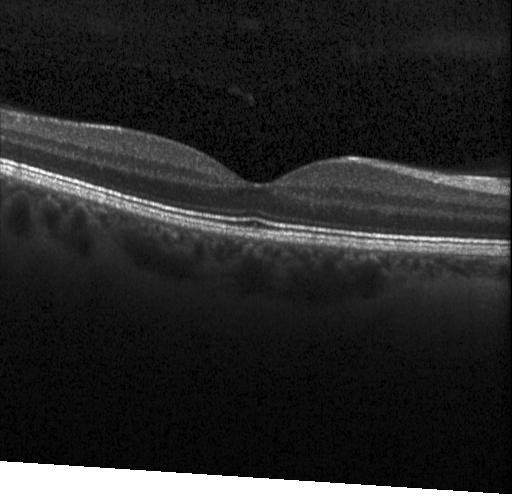 No evidence of CNV, DME, or drusen.